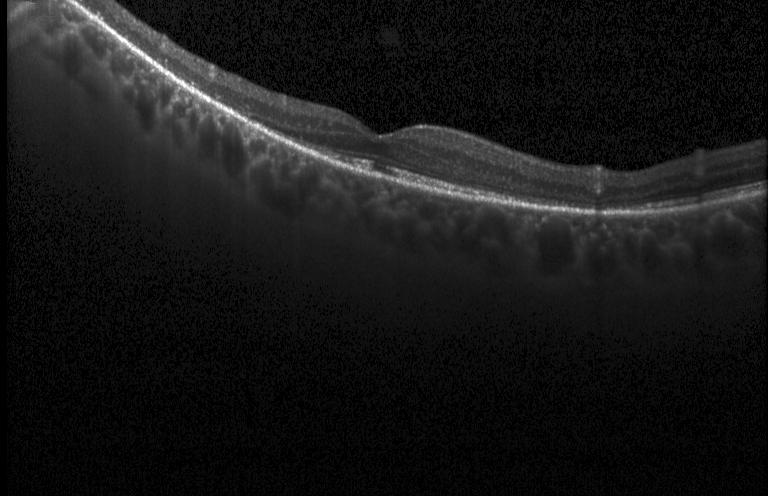

OCT B-scan — Assessment: no CNV, no DME, and no drusen.